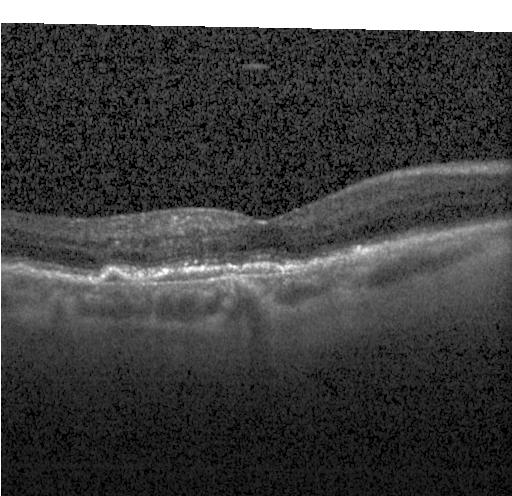
Optical coherence tomography scan — Impression: a choroidal neovascular membrane.